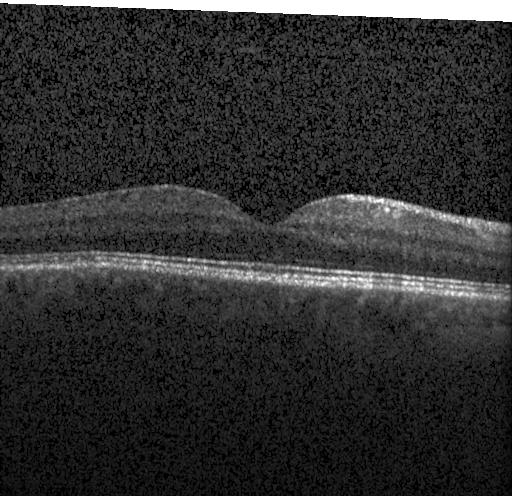
Macular OCT: no choroidal neovascularization, diabetic macular edema, or drusen.